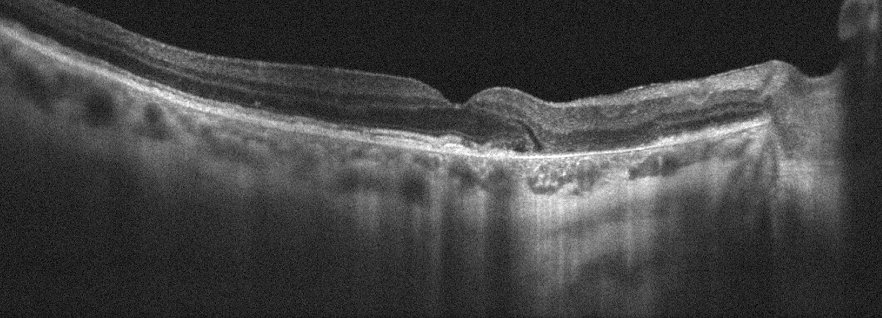

Acquired on an Optovue Avanti RTVue XR. Fovea-centered. OCT line scan
Macular OCT: AMD.